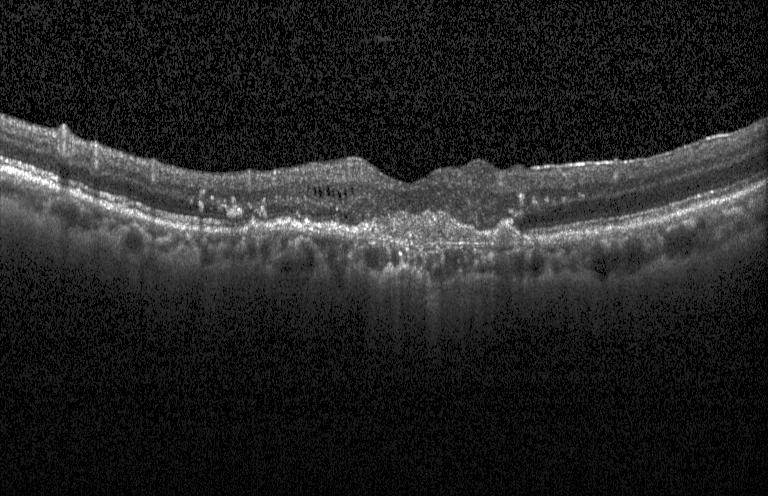 Through the macula; instrument: Heidelberg Spectralis; retinal OCT cross-section
Diagnosis: choroidal neovascularization (CNV).